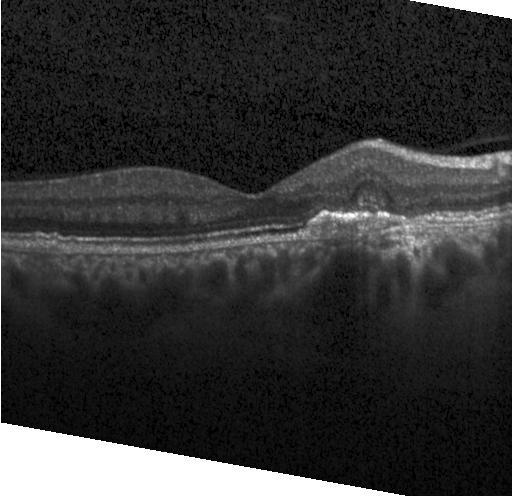

OCT B-scan; centered on the fovea; spectral-domain optical coherence tomography; Heidelberg Spectralis OCT system.
Impression: a choroidal neovascular membrane.